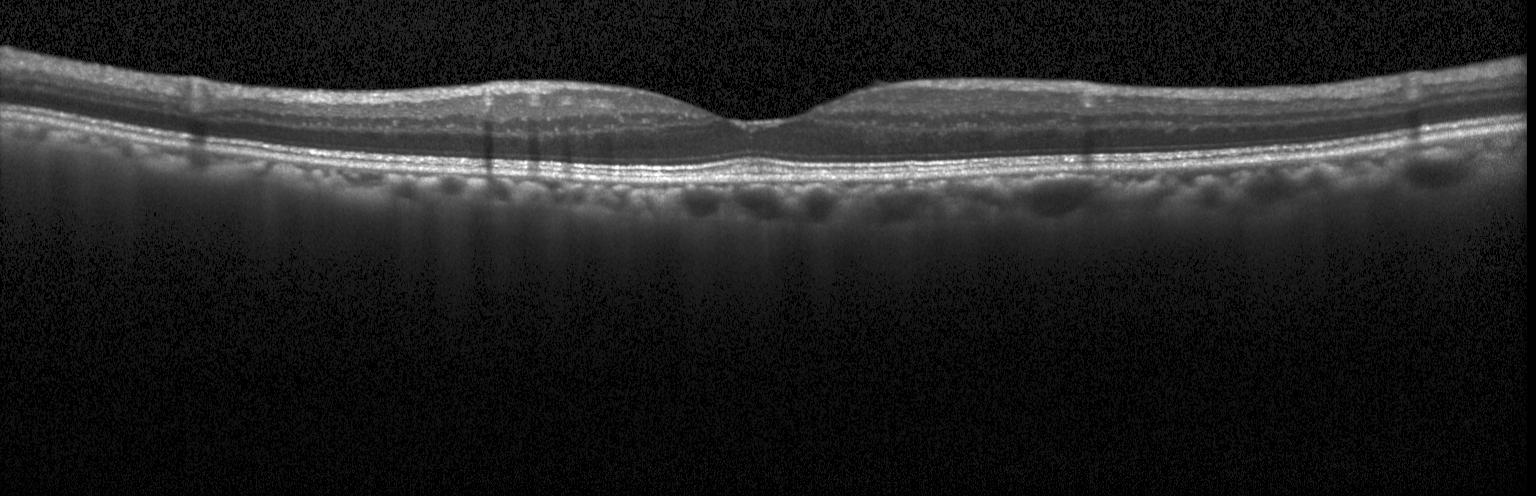 Finding: no evidence of choroidal neovascularization, diabetic macular edema, or drusen.